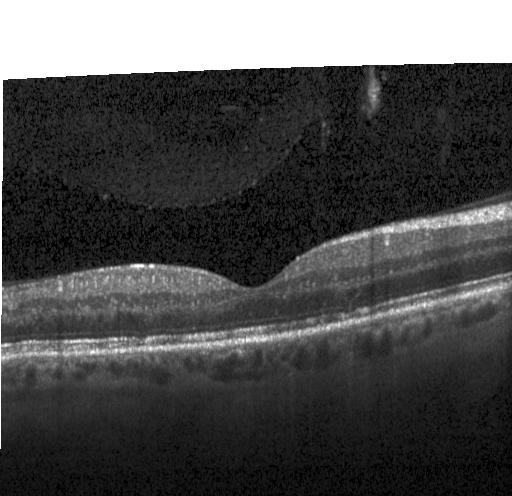
SD-OCT · OCT line scan · centered on the fovea · instrument: Heidelberg Spectralis.
Dx: neither CNV, DME, nor drusen.